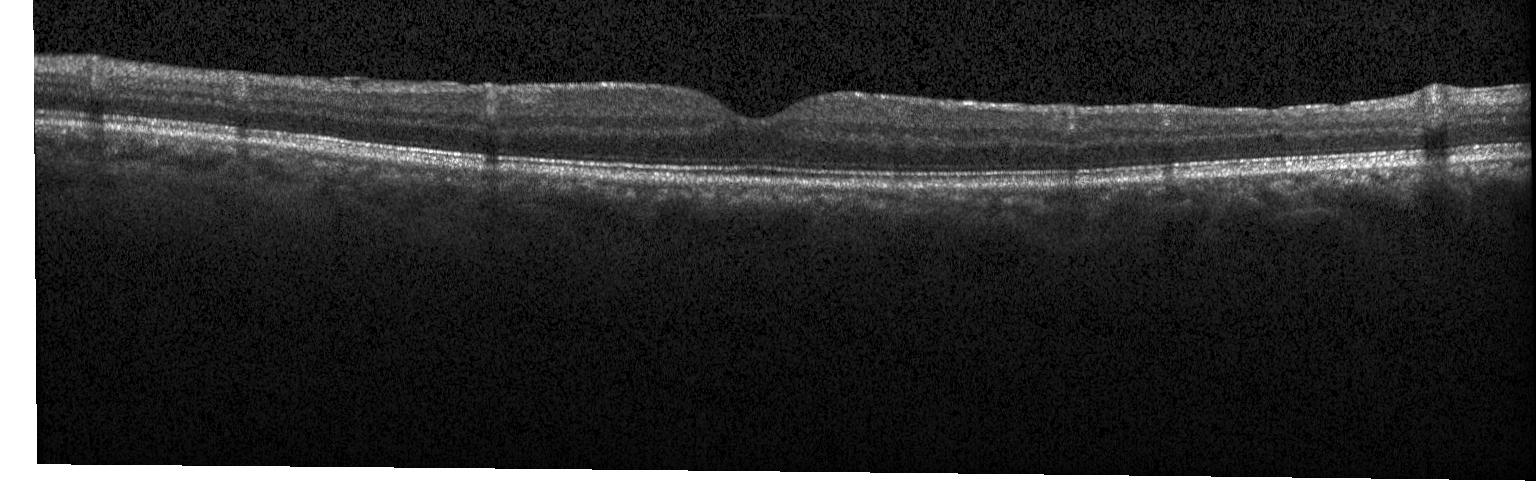 OCT line scan. No CNV, no DME, and no drusen.